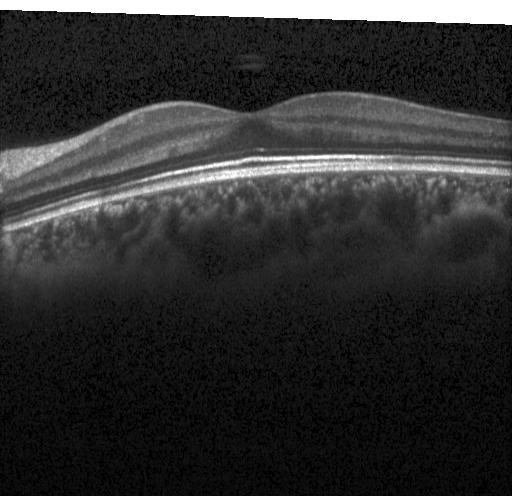

Finding: no choroidal neovascularization, no diabetic macular edema, and no drusen.